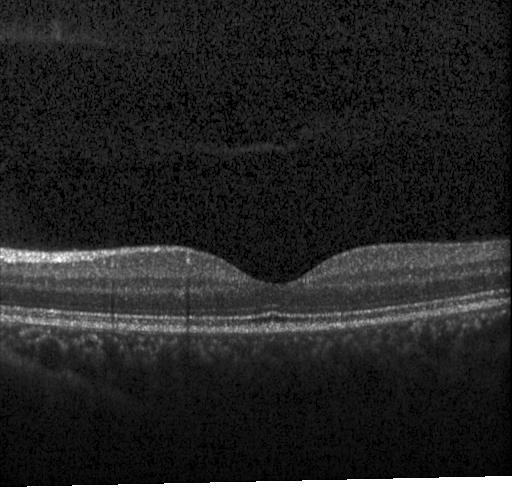

Macular OCT: no choroidal neovascularization, diabetic macular edema, or drusen.